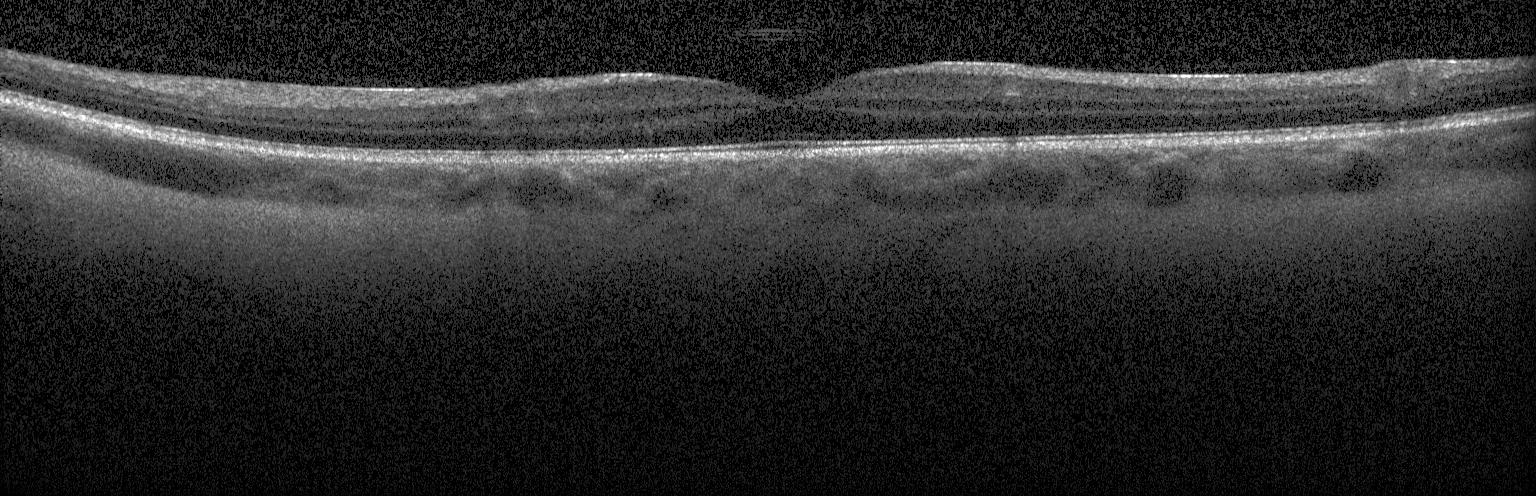 Retinal OCT B-scan. Macular OCT: no evidence of CNV, DME, or drusen.